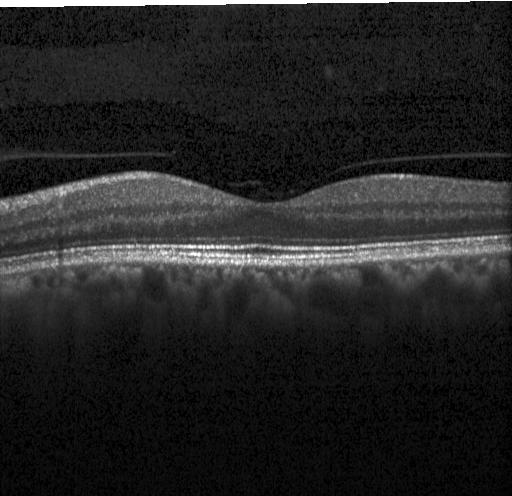

Optical coherence tomography B-scan. Macular OCT: no choroidal neovascularization, diabetic macular edema, or drusen.